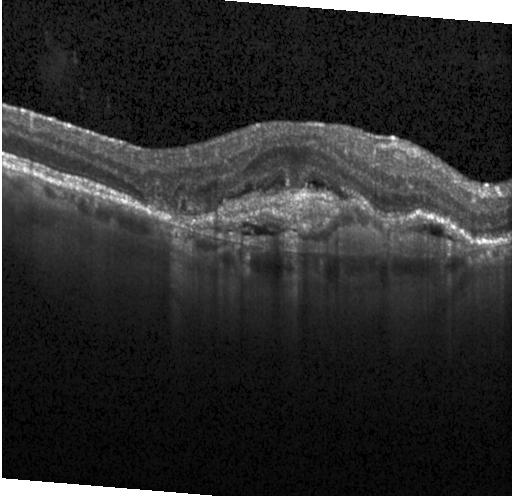
OCT line scan · horizontal scan through the fovea. OCT finding: CNV.